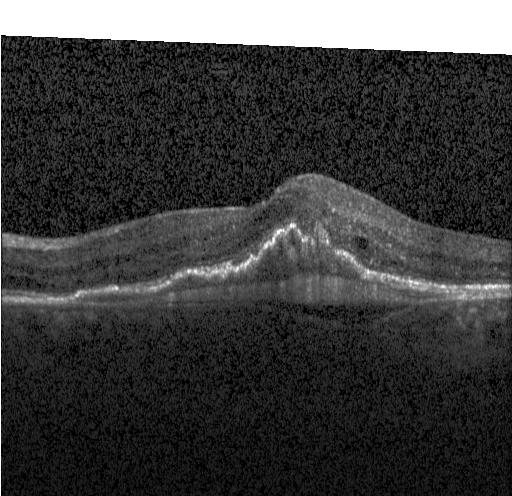
OCT B-scan. Impression: a choroidal neovascular membrane.